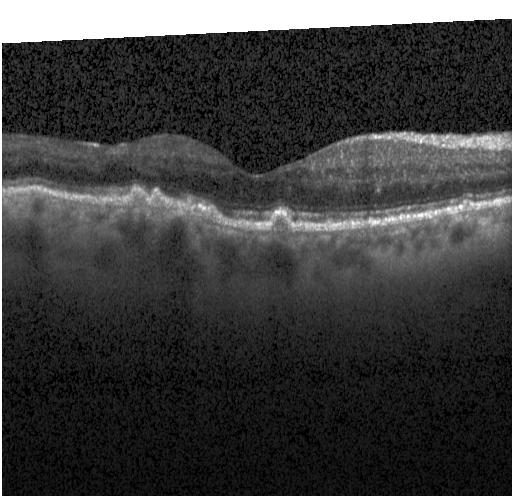 OCT B-scan showing multiple drusen.